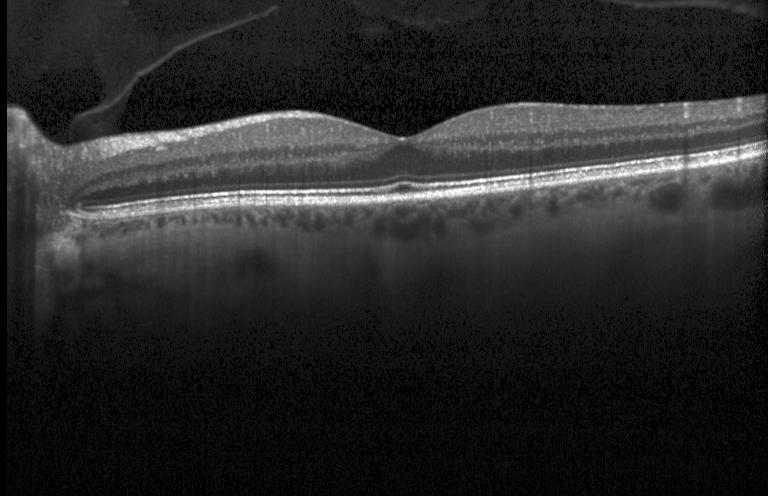 Macular OCT: no choroidal neovascularization, no diabetic macular edema, and no drusen.